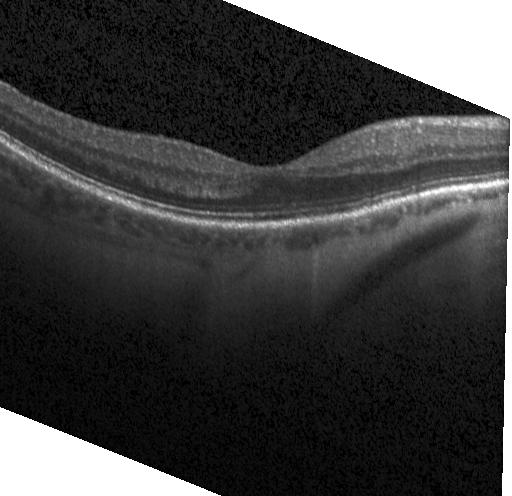
Retinal OCT cross-section
Impression: no choroidal neovascularization, no diabetic macular edema, and no drusen.